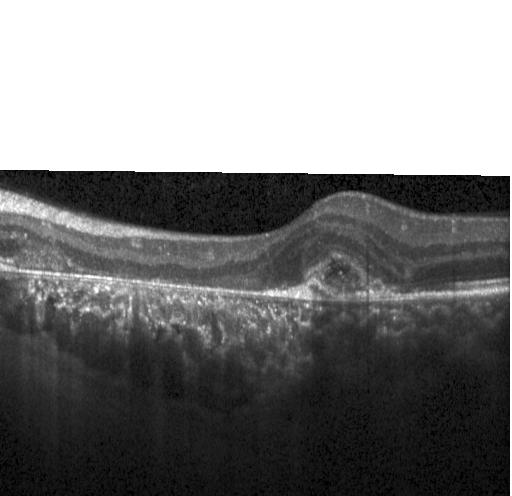
Choroidal neovascularization (CNV).